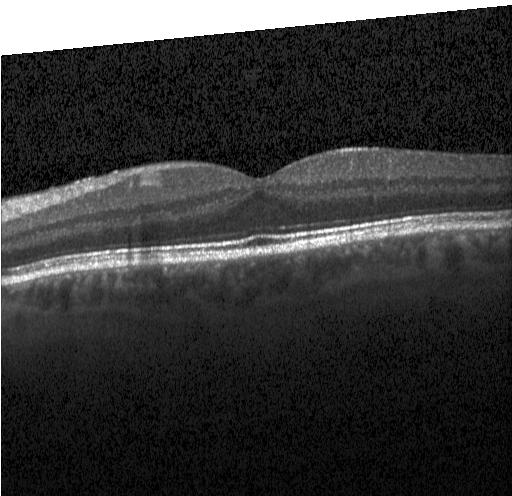

OCT B-scan.
Diagnosis: no choroidal neovascularization, no diabetic macular edema, and no drusen.